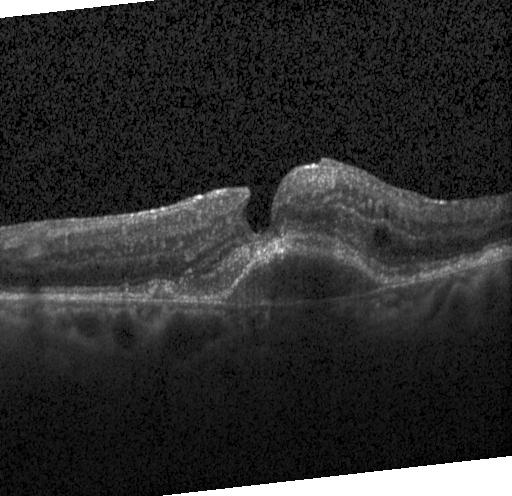

Finding: a choroidal neovascular membrane.